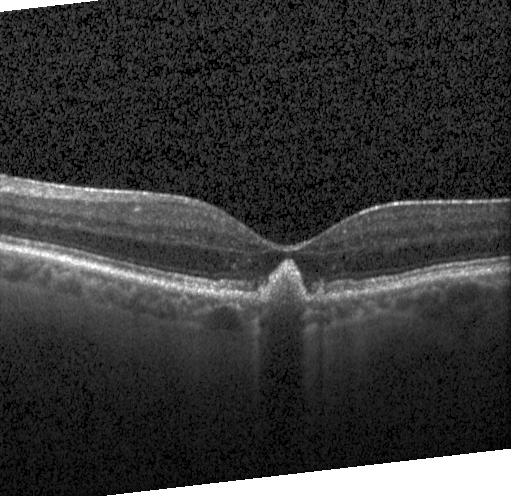 Diagnosis: choroidal neovascularization (CNV).